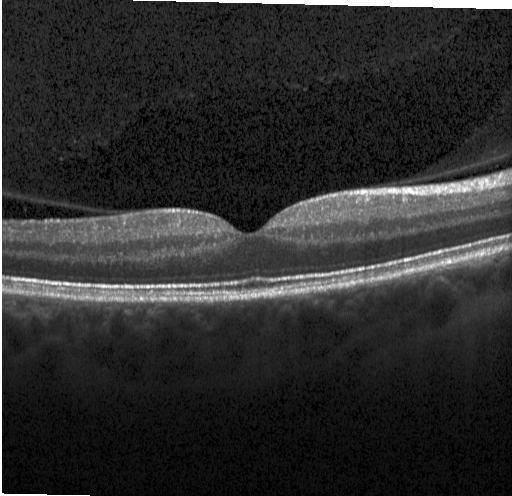 OCT line scan.
Impression: neither CNV, DME, nor drusen.